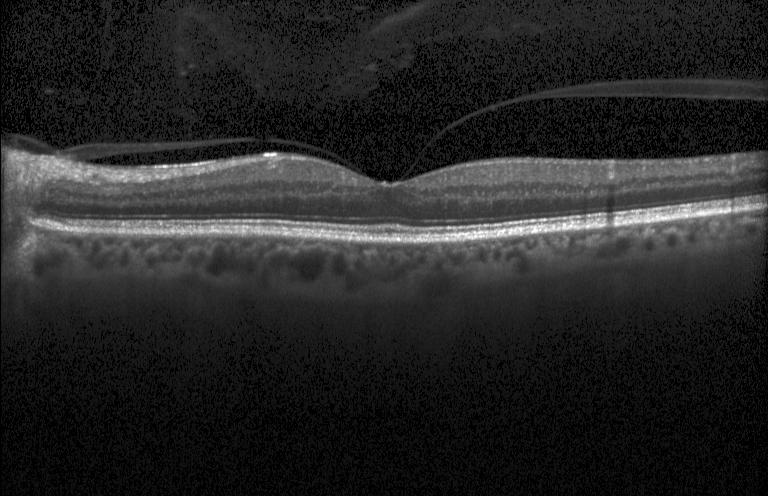
Dx: no evidence of CNV, DME, or drusen.